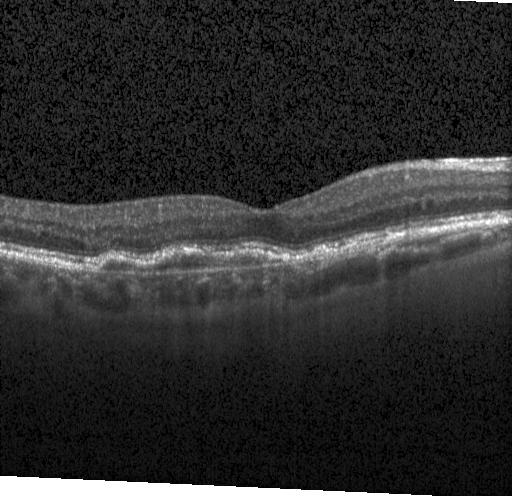 OCT B-scan
Diagnosis: choroidal neovascularization.